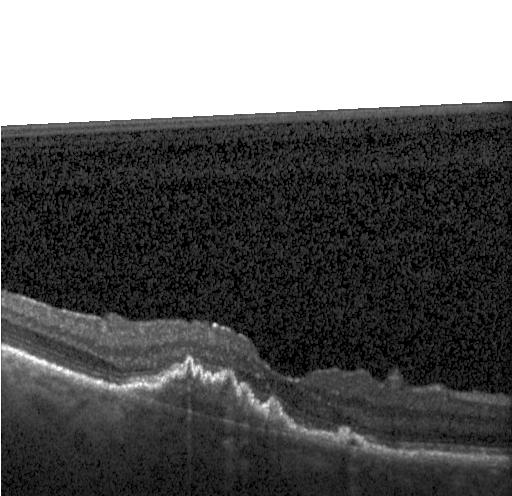
The scan shows choroidal neovascularization.